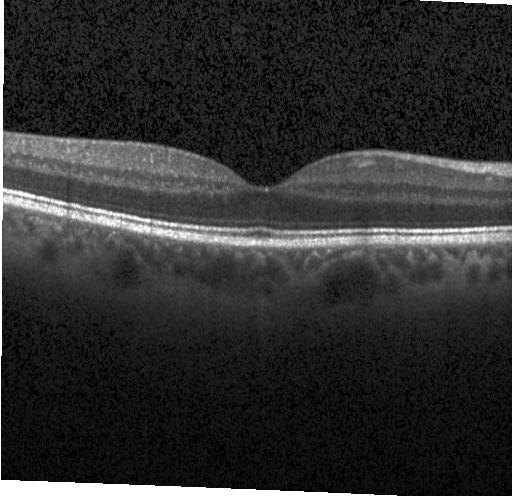 OCT line scan; SD-OCT. Diagnosis: no CNV, no DME, and no drusen.